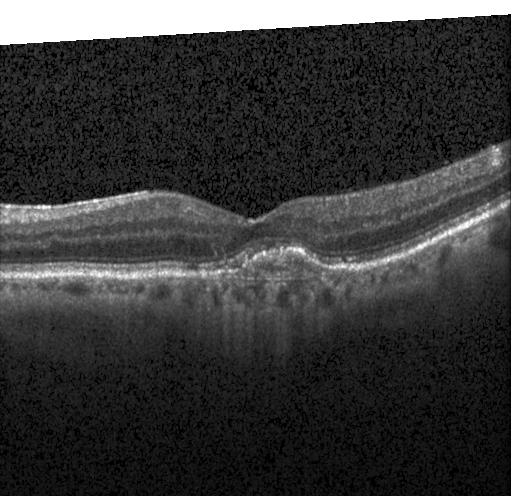 Dx: a choroidal neovascular membrane.